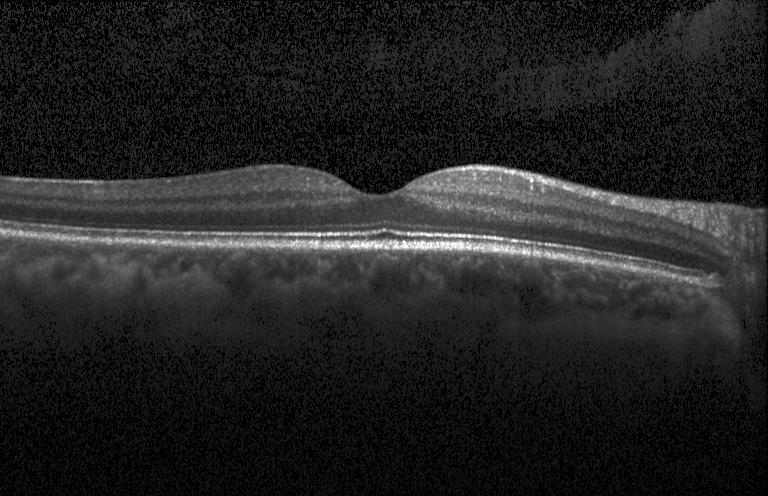

OCT finding: no evidence of choroidal neovascularization, diabetic macular edema, or drusen.